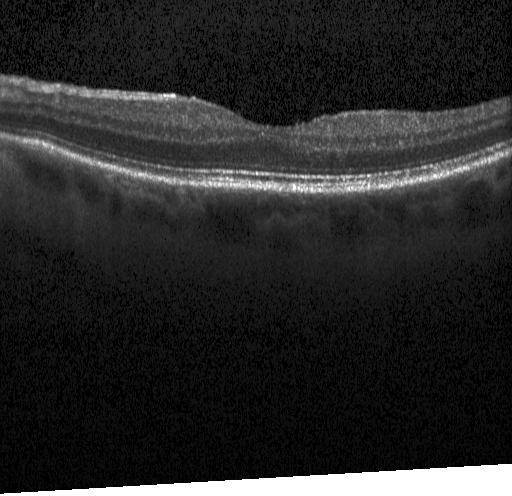
Dx: no evidence of choroidal neovascularization, diabetic macular edema, or drusen.